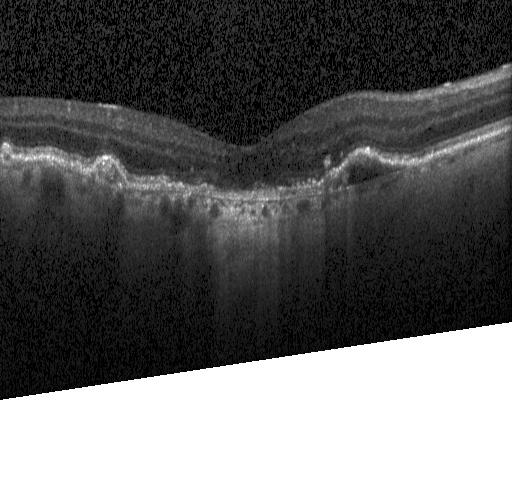
Instrument: Heidelberg Spectralis; OCT B-scan — The scan shows choroidal neovascularization.